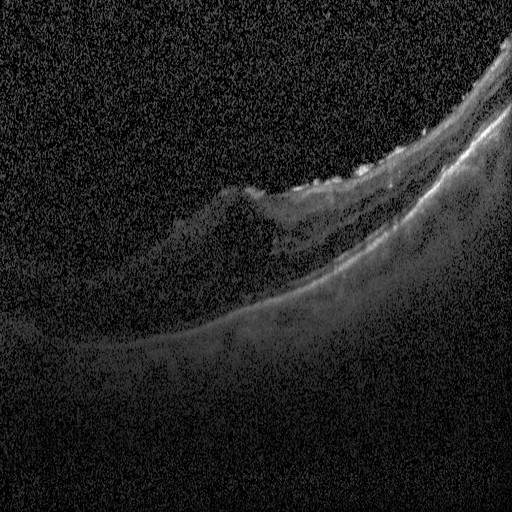

This B-scan demonstrates diabetic macular edema.